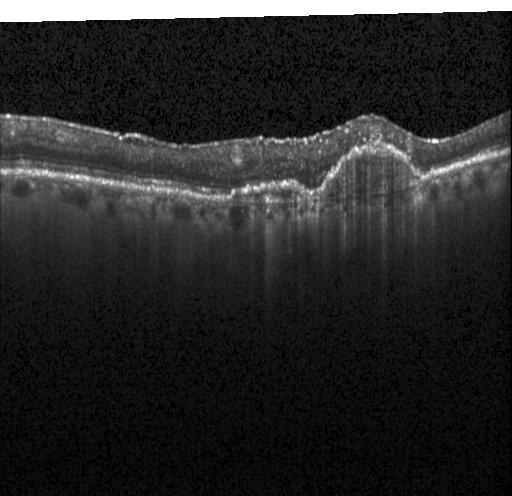
OCT B-scan showing a choroidal neovascular membrane.